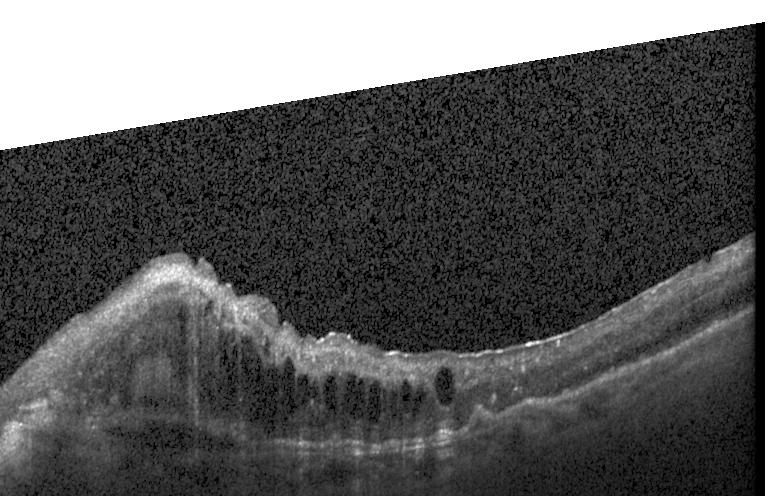

Dx: CNV.